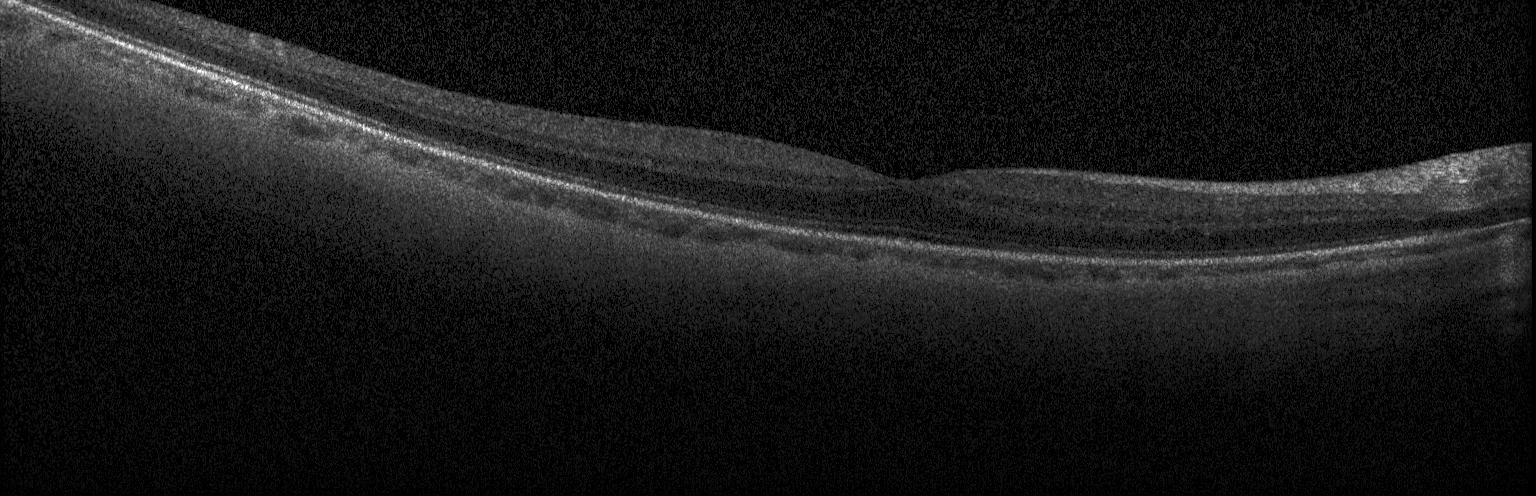
Optical coherence tomography B-scan · SD-OCT · through the macula · acquired on a Heidelberg Spectralis. Diagnosis: no evidence of choroidal neovascularization, diabetic macular edema, or drusen.